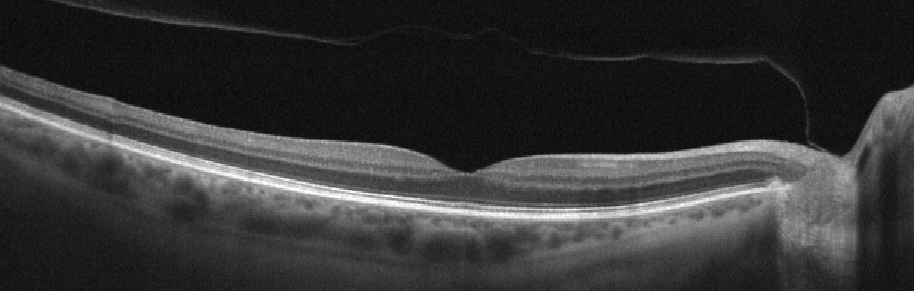
OCT B-scan · right eye. Macular OCT: absence of AMD, DME, ERM, RAO, RVO, and vitreomacular interface disease.